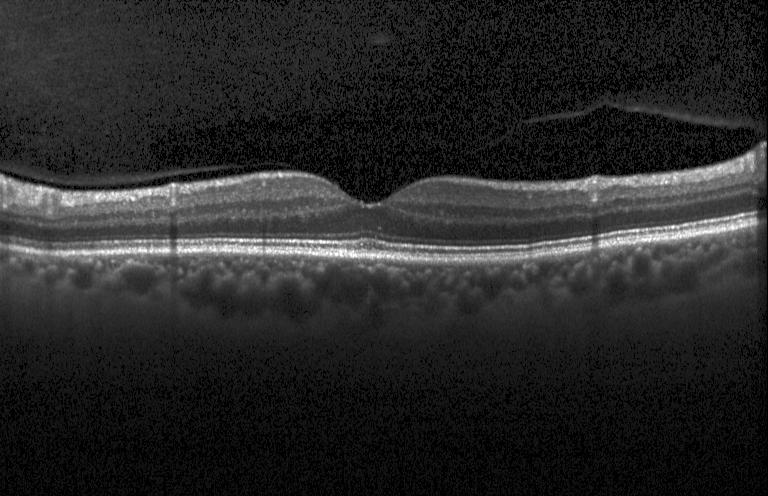
Retinal OCT B-scan — Dx: neither CNV, DME, nor drusen.